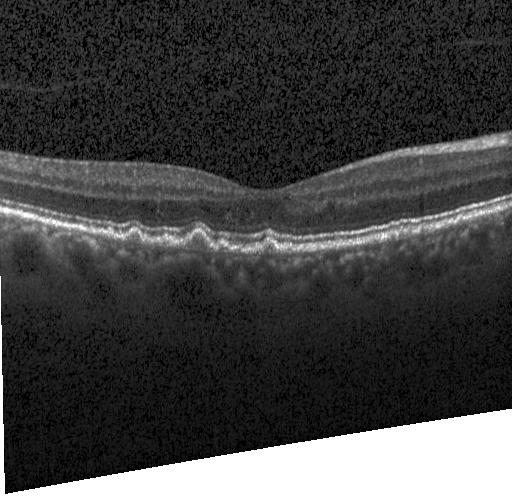

Retinal OCT cross-section; spectral-domain optical coherence tomography; instrument: Heidelberg Spectralis — The scan shows sub-RPE drusenoid deposits.